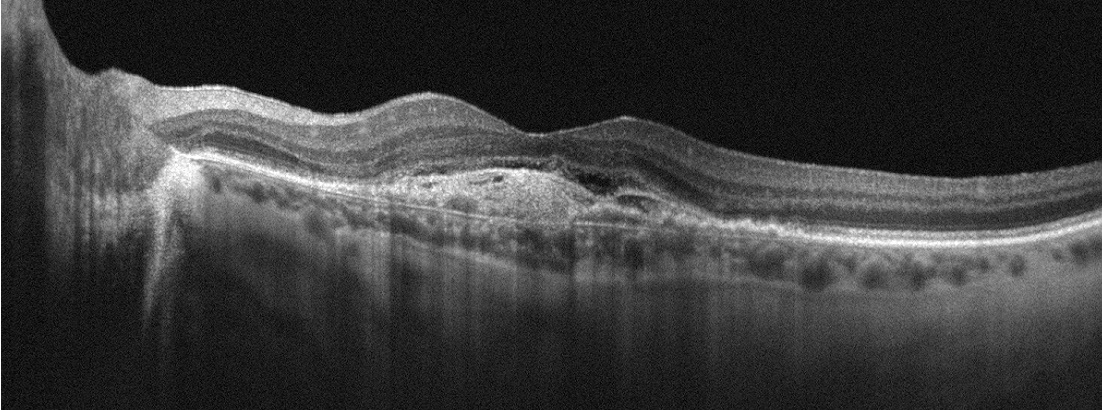 Retinal OCT cross-section, fovea-centered — Macular OCT: AMD.